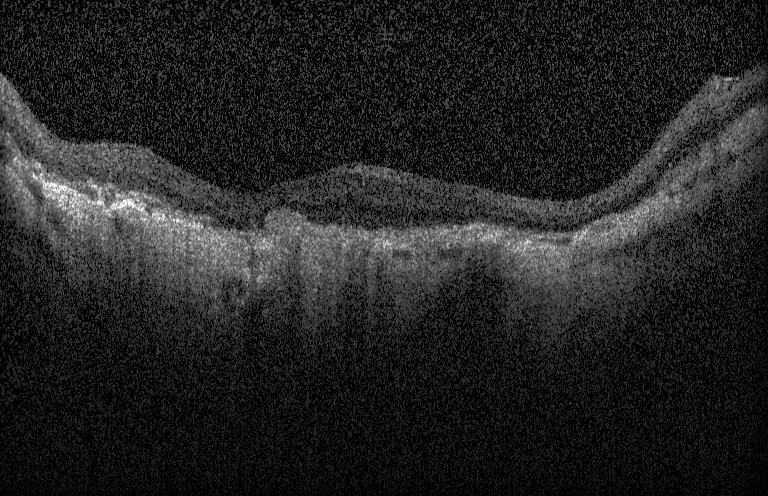

Dx: a choroidal neovascular membrane.